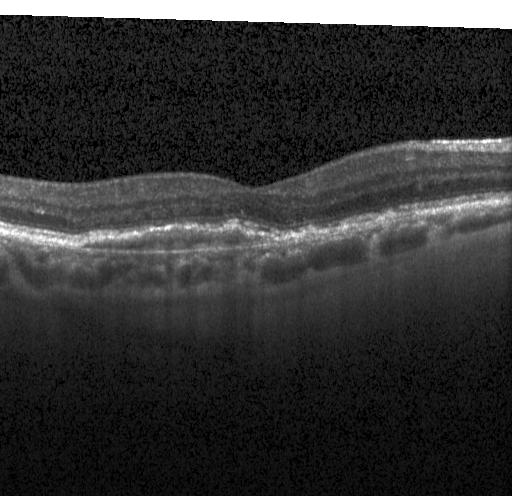 Retinal OCT B-scan · spectral-domain OCT
Diagnosis: a choroidal neovascular membrane.